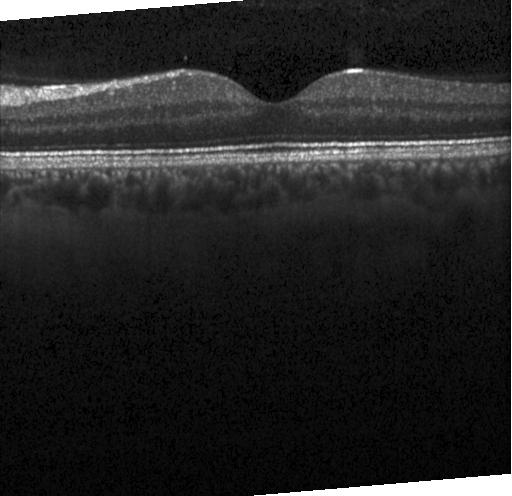 Retinal OCT cross-section.
Impression: no evidence of CNV, DME, or drusen.